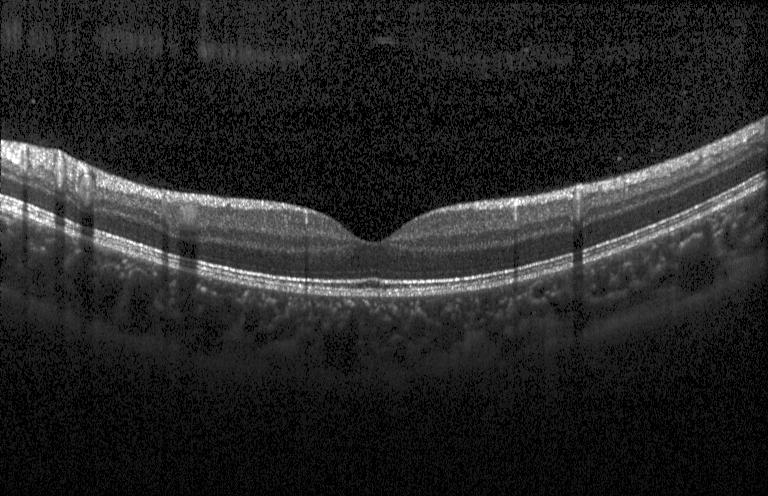

OCT B-scan — Neither CNV, DME, nor drusen.